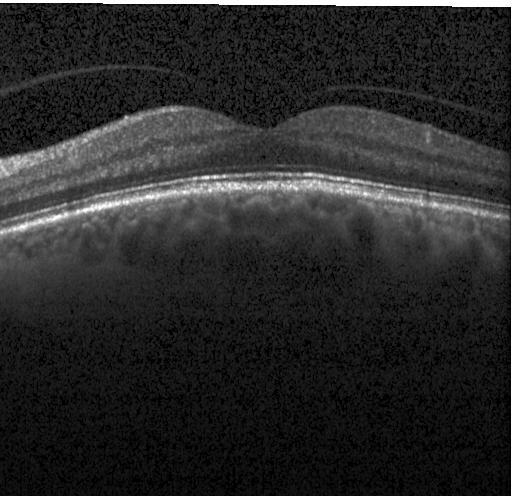 SD-OCT · instrument: Heidelberg Spectralis · retinal OCT cross-section — Macular OCT: no choroidal neovascularization, diabetic macular edema, or drusen.